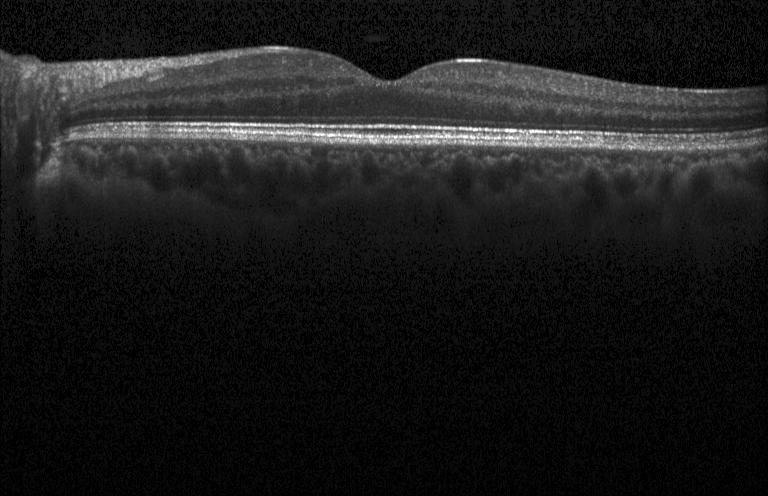

Optical coherence tomography scan, spectral-domain optical coherence tomography, horizontal scan through the fovea.
Macular OCT: no choroidal neovascularization, diabetic macular edema, or drusen.